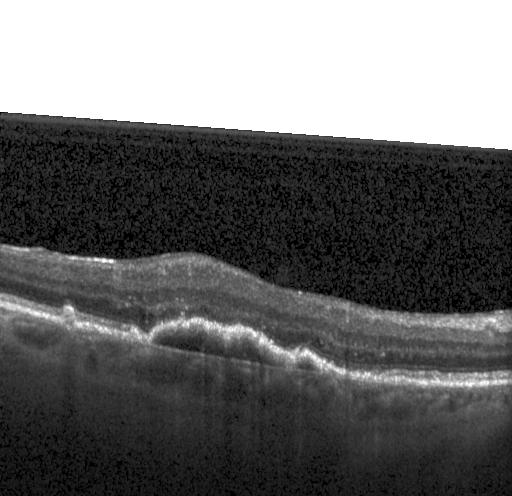
OCT line scan
Finding: choroidal neovascularization.